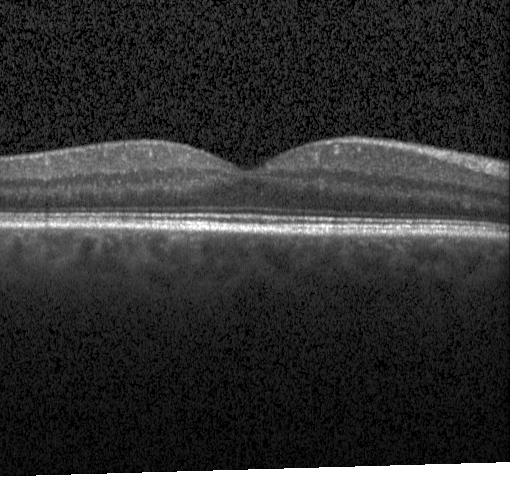

Through the macula; optical coherence tomography scan.
Assessment: no evidence of choroidal neovascularization, diabetic macular edema, or drusen.